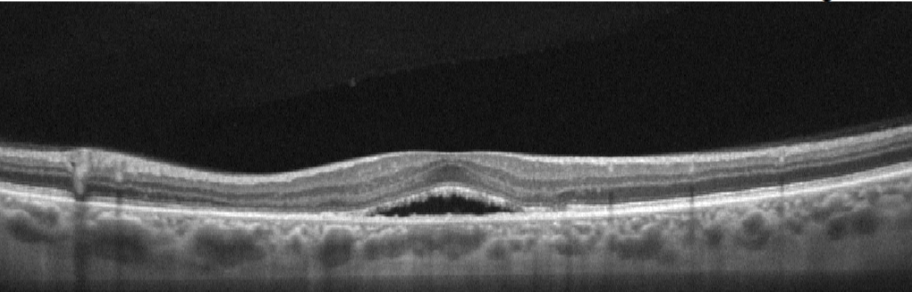
Assessment: age-related macular degeneration.